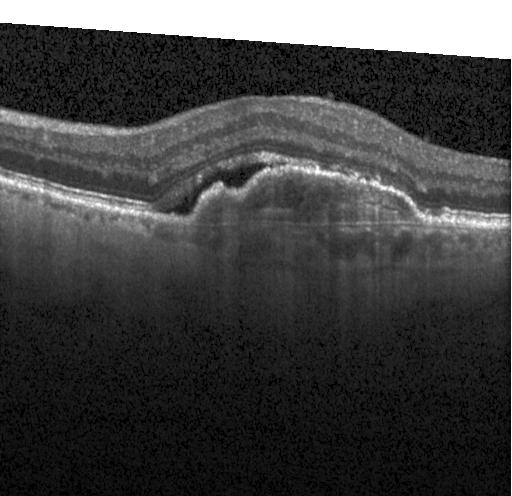
Assessment: a choroidal neovascular membrane.